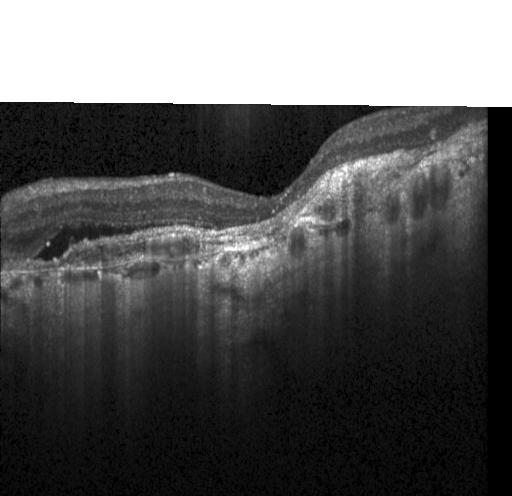 Spectral-domain OCT · OCT B-scan · Heidelberg Spectralis OCT system
OCT finding: choroidal neovascularization (CNV).